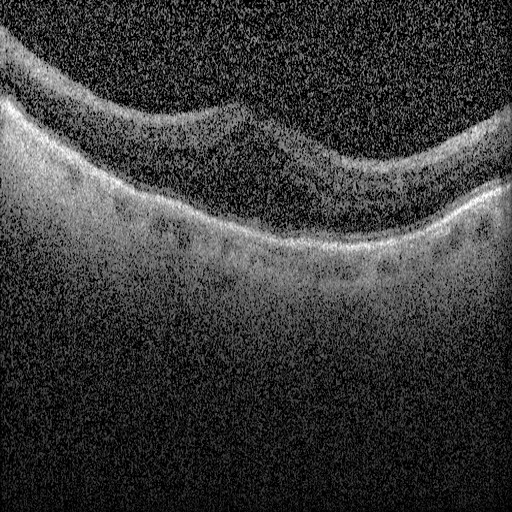 Spectral-domain OCT B-scan: diabetic macular edema (DME).